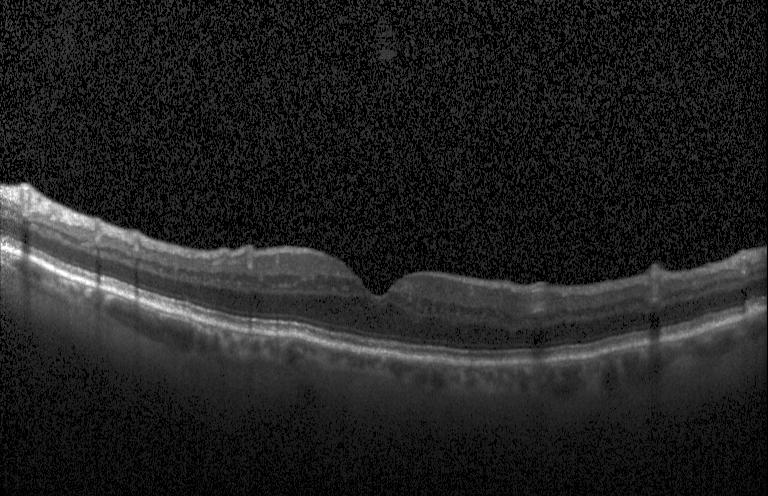

Diagnosis: no choroidal neovascularization, no diabetic macular edema, and no drusen.